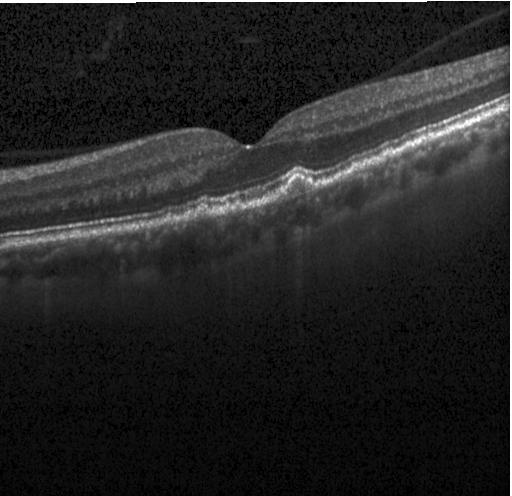 Diagnosis: sub-RPE drusenoid deposits.